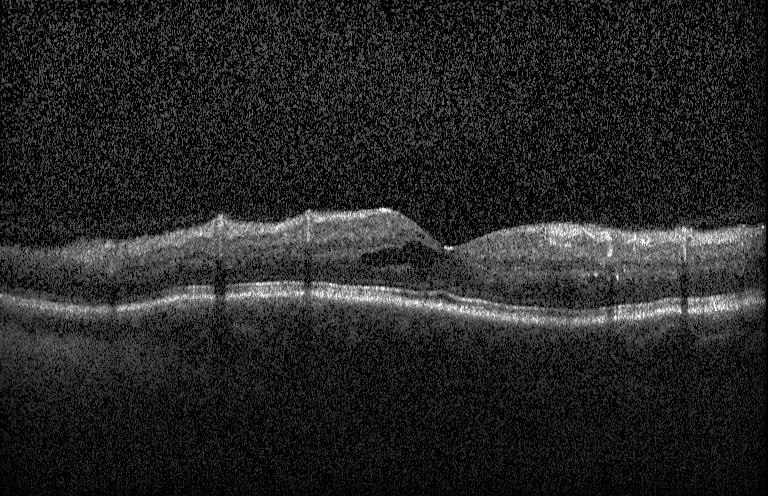
Optical coherence tomography B-scan
OCT finding: DME.